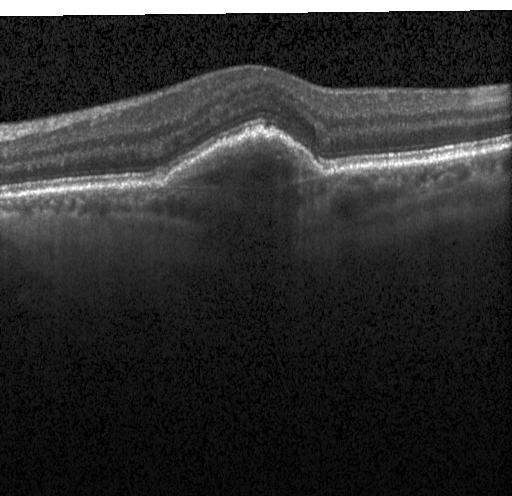
Finding: choroidal neovascularization.